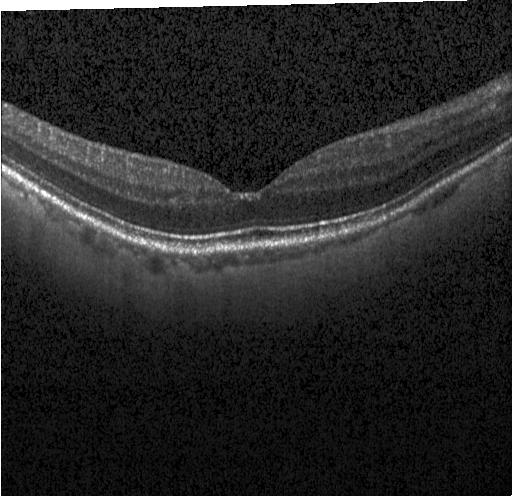

The scan shows no evidence of CNV, DME, or drusen.